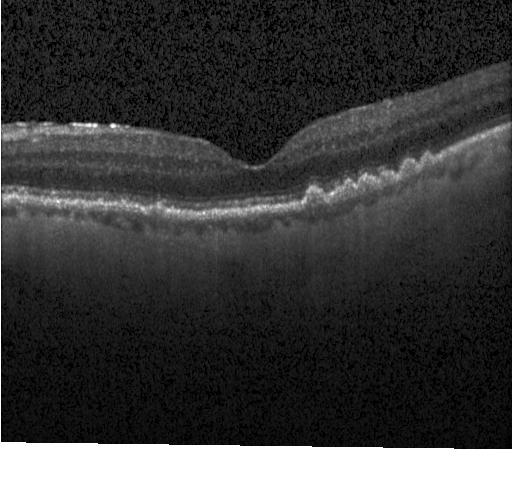

Retinal OCT B-scan — Macular OCT: multiple drusen.